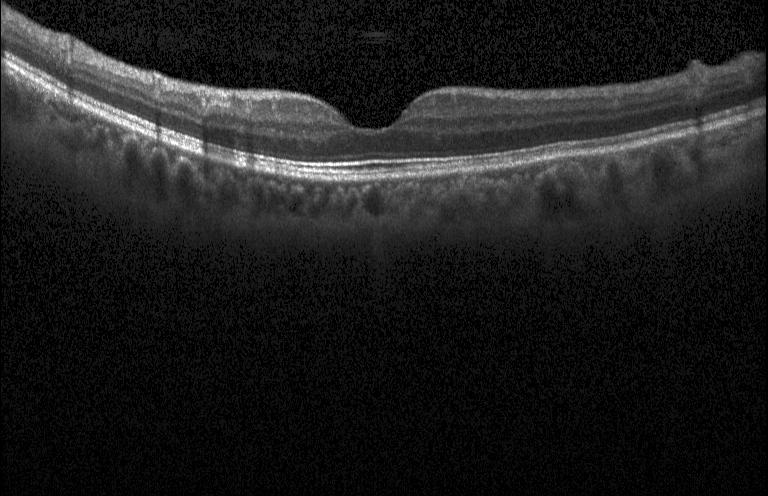 Impression: no choroidal neovascularization, no diabetic macular edema, and no drusen.